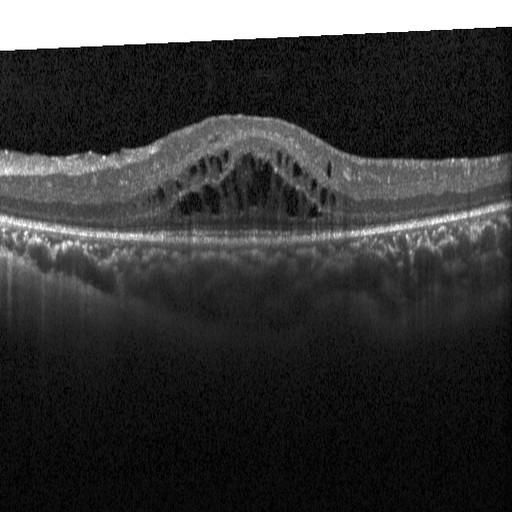 The scan shows DME.